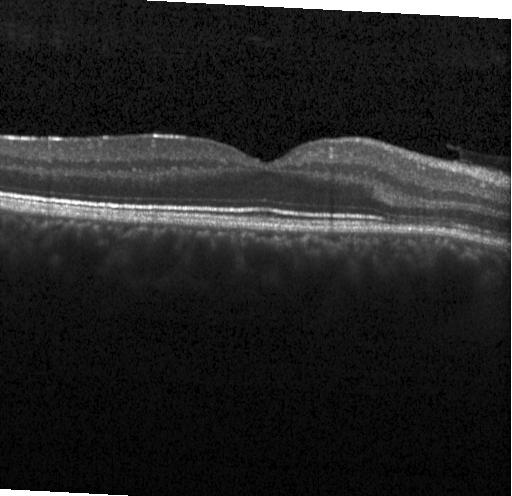 Macular scan, spectral-domain OCT, acquired on a Heidelberg Spectralis, optical coherence tomography B-scan. Finding: no CNV, DME, or drusen.